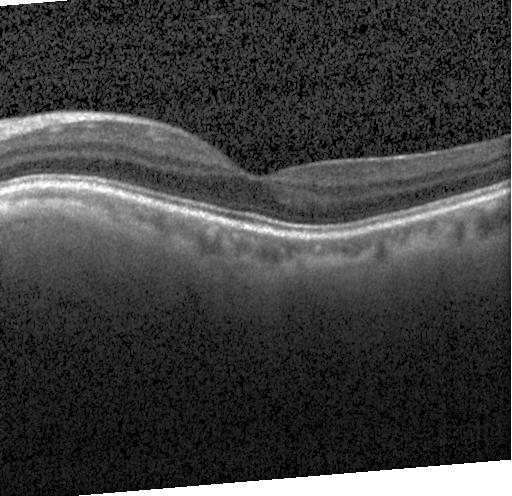
OCT line scan, horizontal scan through the fovea — Macular OCT: neither CNV, DME, nor drusen.